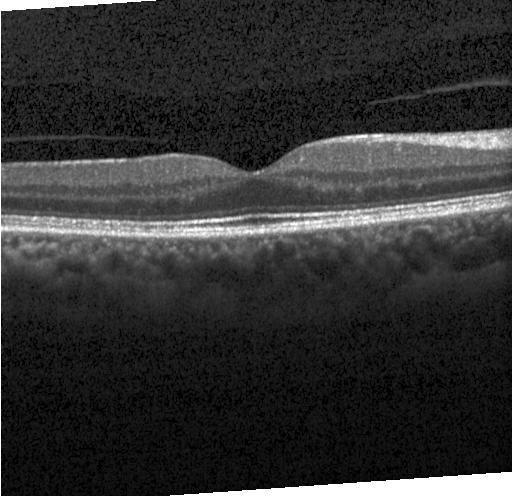 Retinal OCT B-scan; acquired on a Heidelberg Spectralis; fovea-centered
Macular OCT: no choroidal neovascularization, no diabetic macular edema, and no drusen.